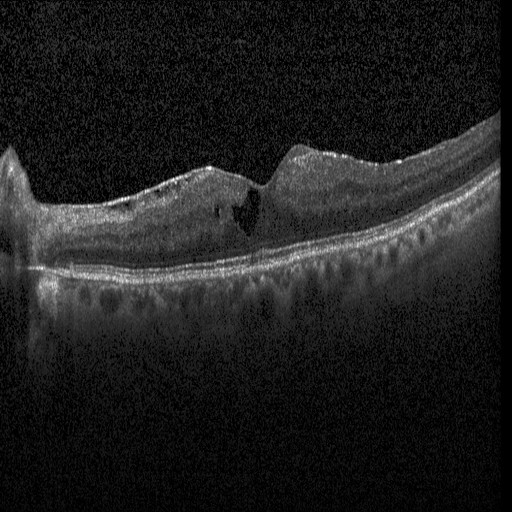

SD-OCT; acquired on a Heidelberg Spectralis; OCT B-scan; macular scan. Impression: diabetic macular edema (DME).